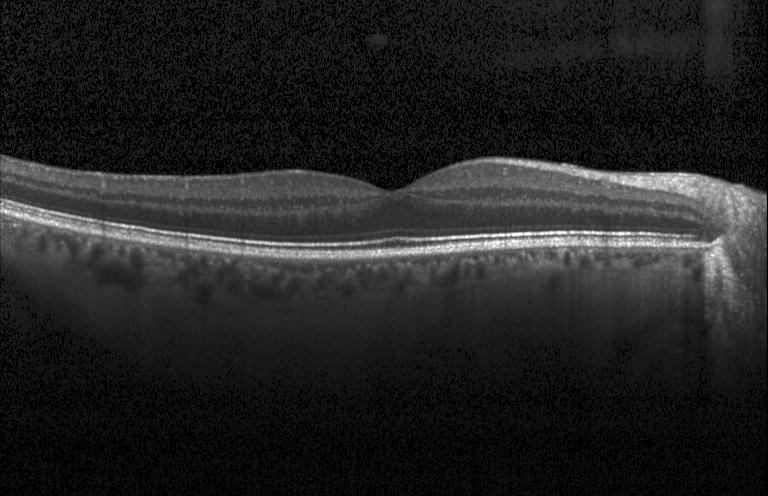

Heidelberg Spectralis OCT system. SD-OCT. Optical coherence tomography B-scan. Diagnosis: no evidence of CNV, DME, or drusen.